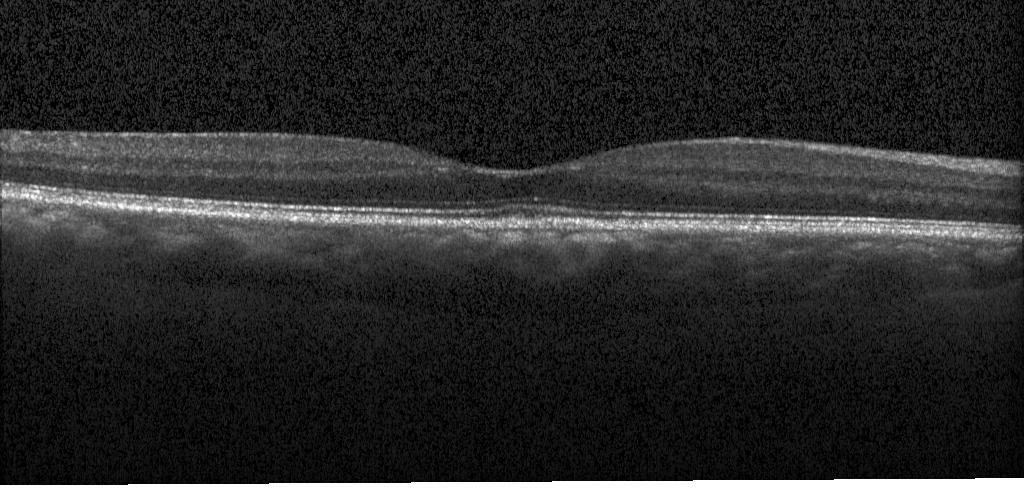 OCT finding: no CNV, no DME, and no drusen.